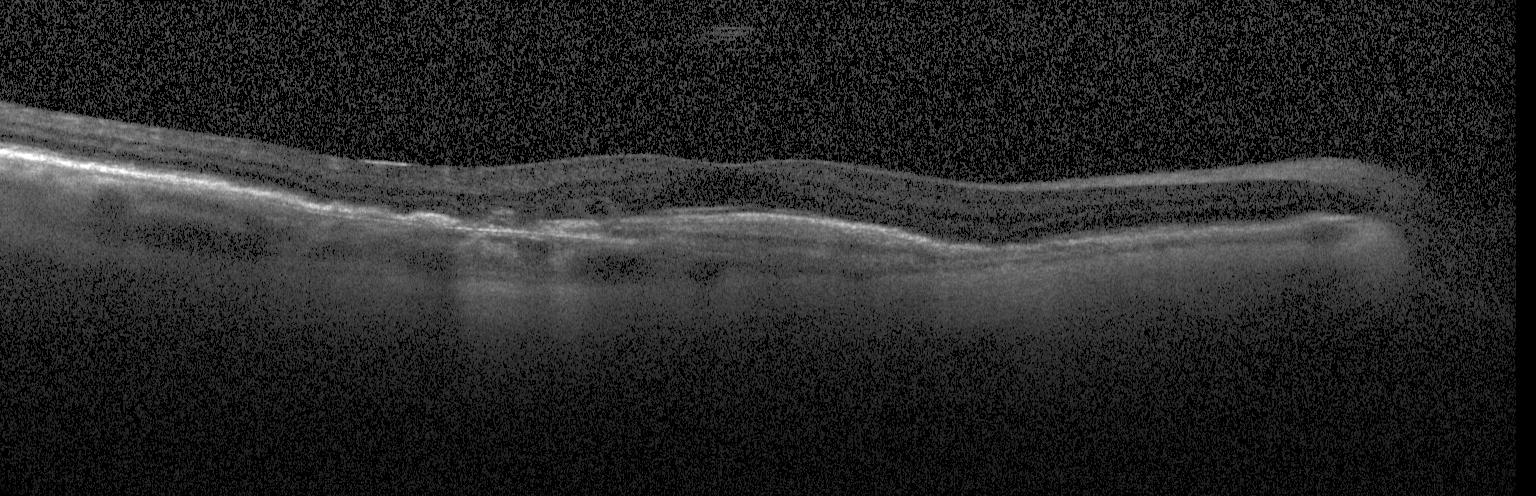
Macular OCT: a choroidal neovascular membrane.